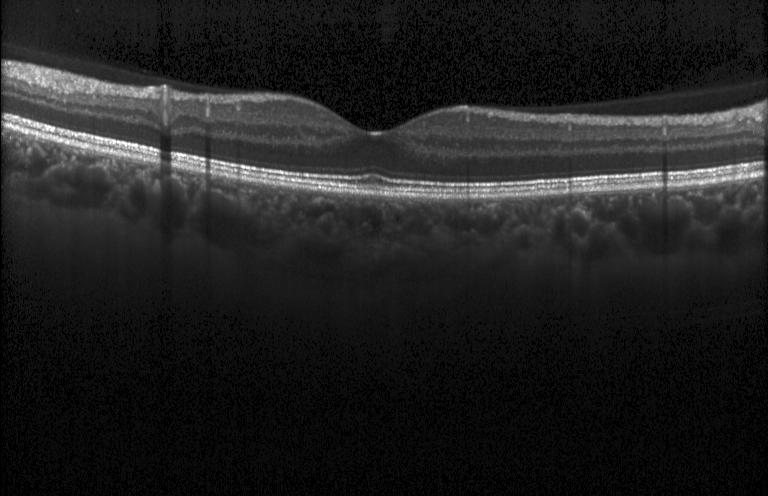

Retinal OCT cross-section showing no choroidal neovascularization, no diabetic macular edema, and no drusen.